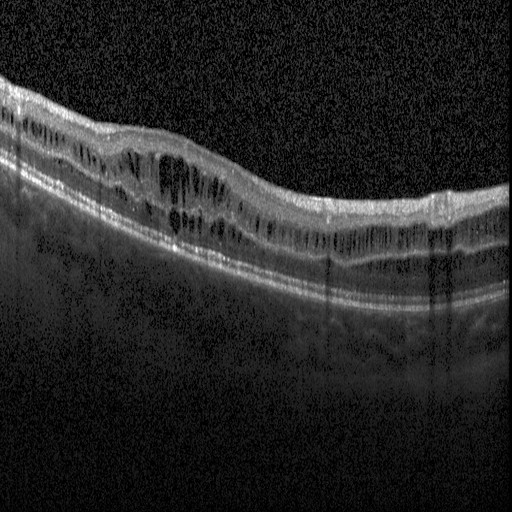

Finding: diabetic macular edema (DME).